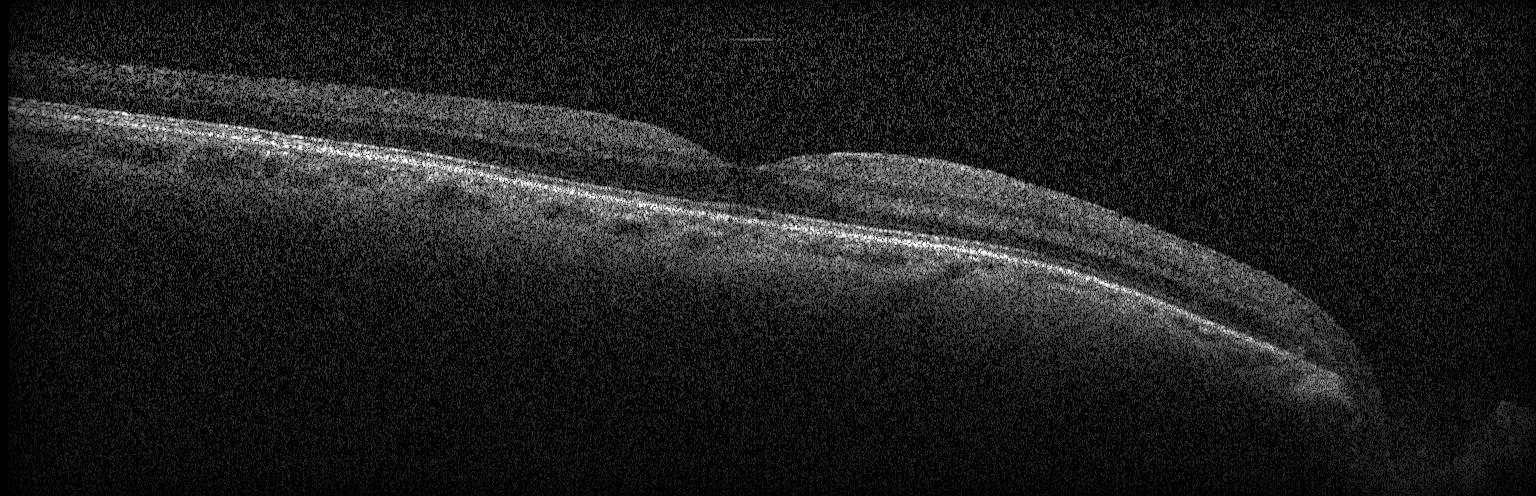
Spectral-domain OCT. Optical coherence tomography B-scan. Fovea-centered.
Finding: no choroidal neovascularization, diabetic macular edema, or drusen.